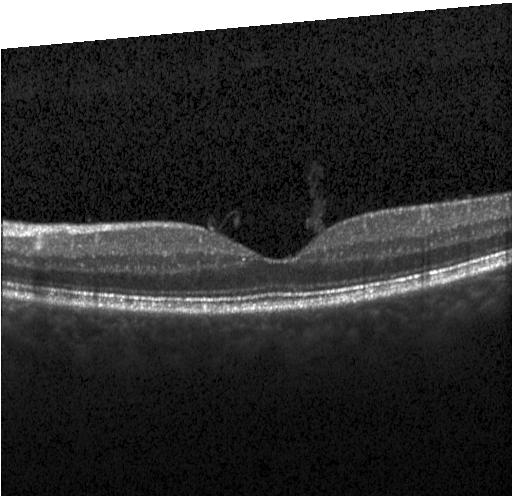

OCT scan showing no evidence of choroidal neovascularization, diabetic macular edema, or drusen.